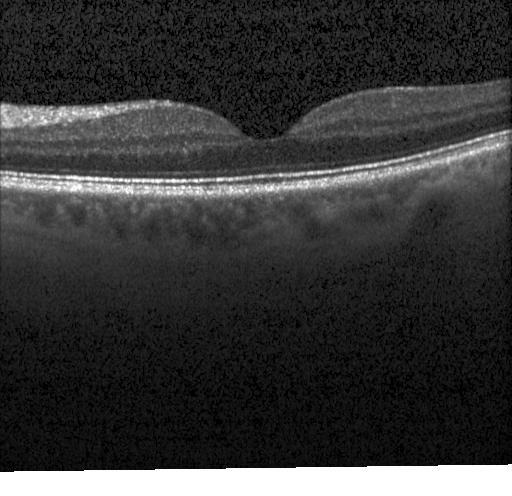

OCT scan showing no CNV, no DME, and no drusen.